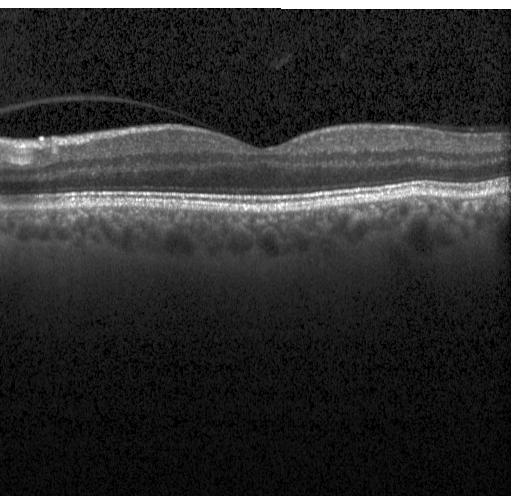

This B-scan demonstrates no evidence of choroidal neovascularization, diabetic macular edema, or drusen.